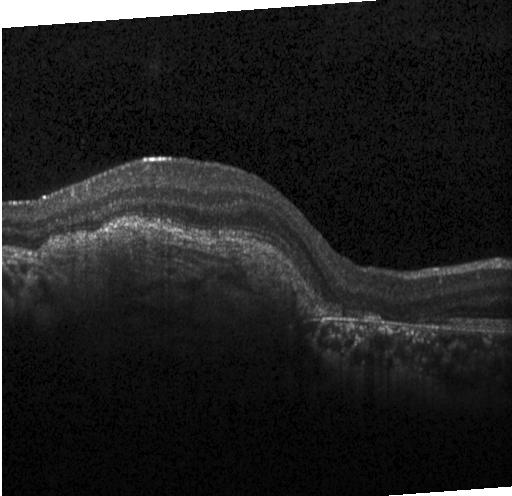 Through the macula · spectral-domain OCT · OCT B-scan — This B-scan demonstrates CNV.